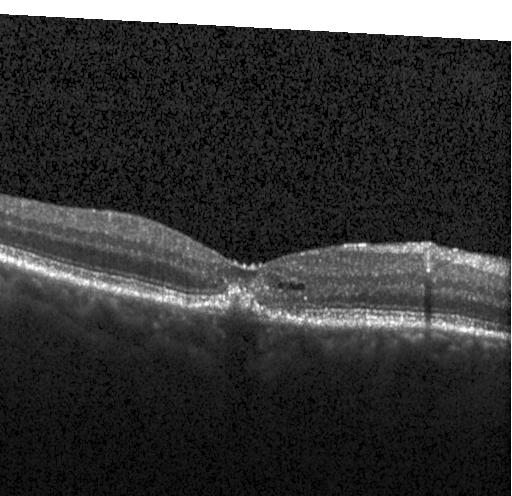
Acquired on a Heidelberg Spectralis. Optical coherence tomography scan. Fovea-centered.
This B-scan demonstrates a choroidal neovascular membrane.